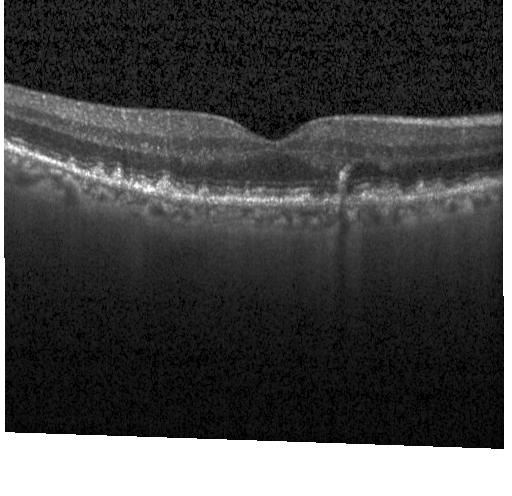
Instrument: Heidelberg Spectralis; OCT B-scan; SD-OCT — Finding: multiple drusen.